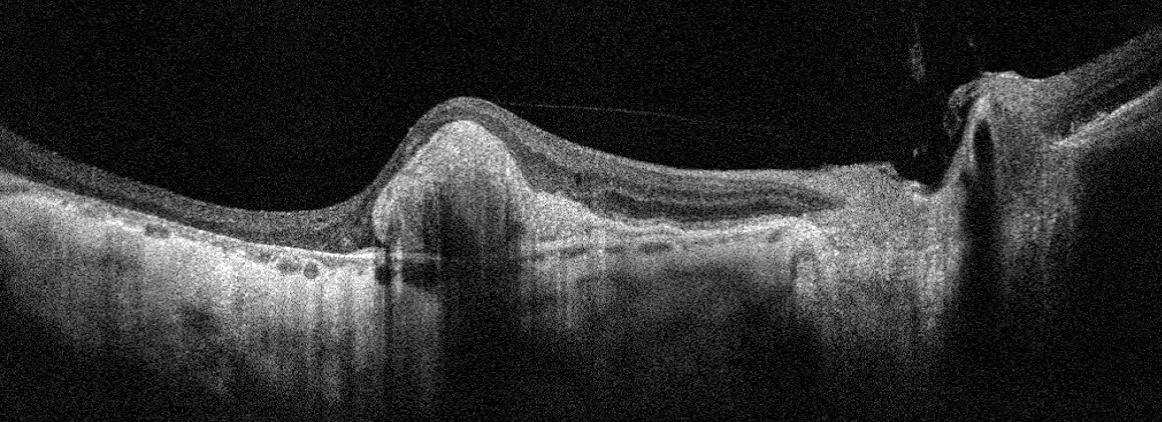
Optovue Avanti RTVue XR · fovea-centered · right eye · retinal OCT B-scan.
Diagnosis: age-related macular degeneration.